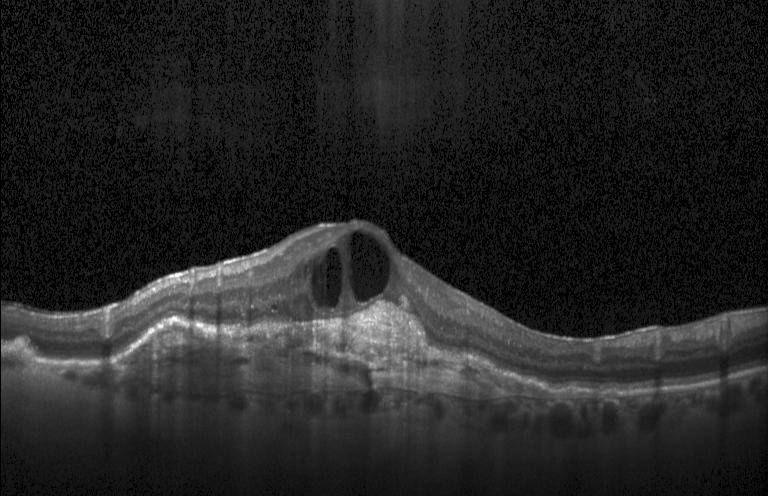 Retinal OCT B-scan. Choroidal neovascularization.